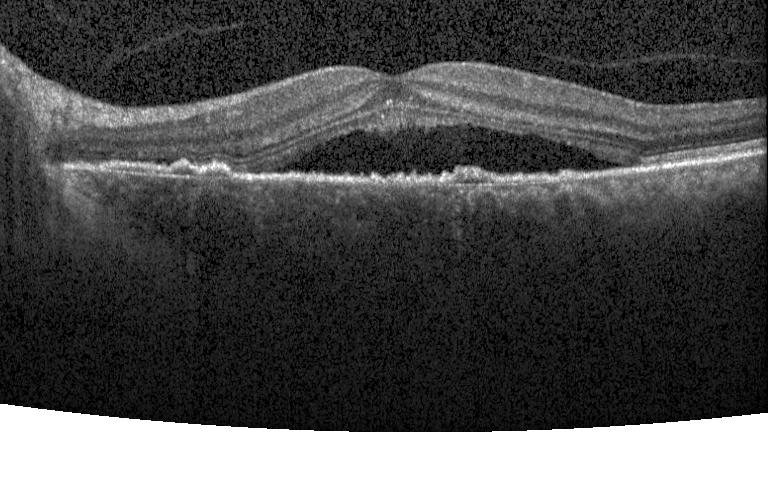

Impression: a choroidal neovascular membrane.